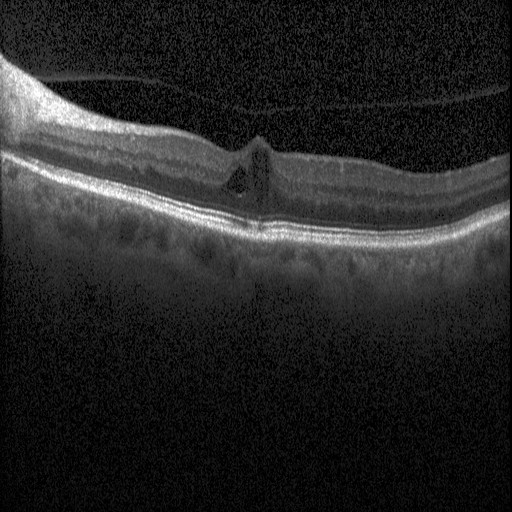

Dx: DME.